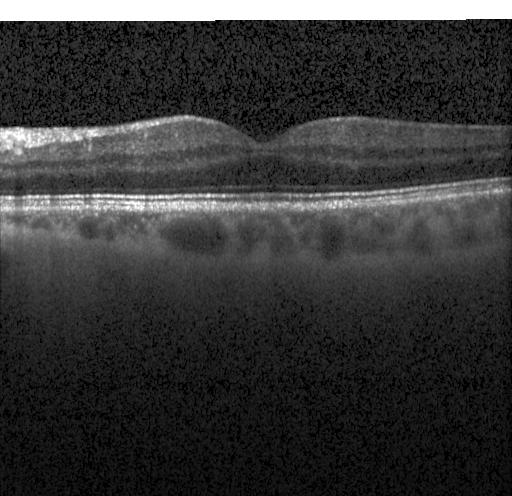 Instrument: Heidelberg Spectralis · spectral-domain OCT · macular scan · optical coherence tomography B-scan
Assessment: no choroidal neovascularization, no diabetic macular edema, and no drusen.